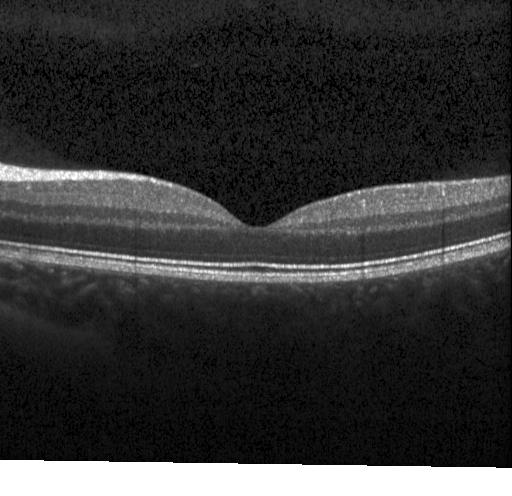 SD-OCT, fovea-centered, OCT line scan.
Dx: no choroidal neovascularization, no diabetic macular edema, and no drusen.